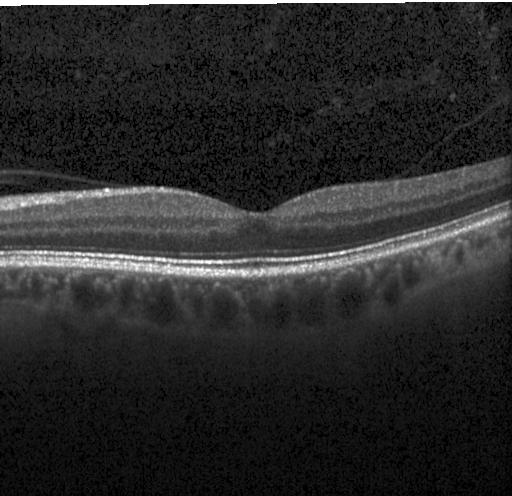 Optical coherence tomography B-scan
The scan shows no choroidal neovascularization, no diabetic macular edema, and no drusen.